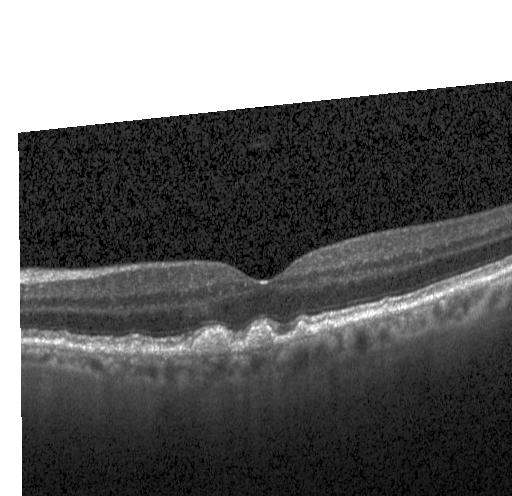
Heidelberg Spectralis, macular scan, retinal OCT cross-section
Finding: drusen.